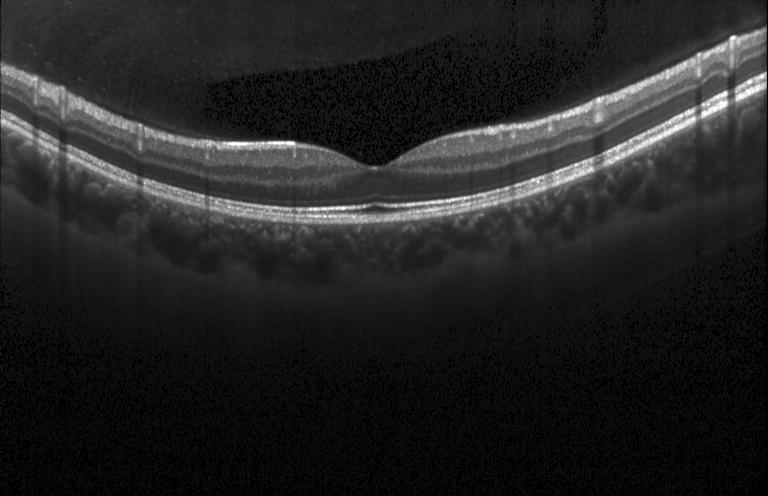 No evidence of choroidal neovascularization, diabetic macular edema, or drusen.